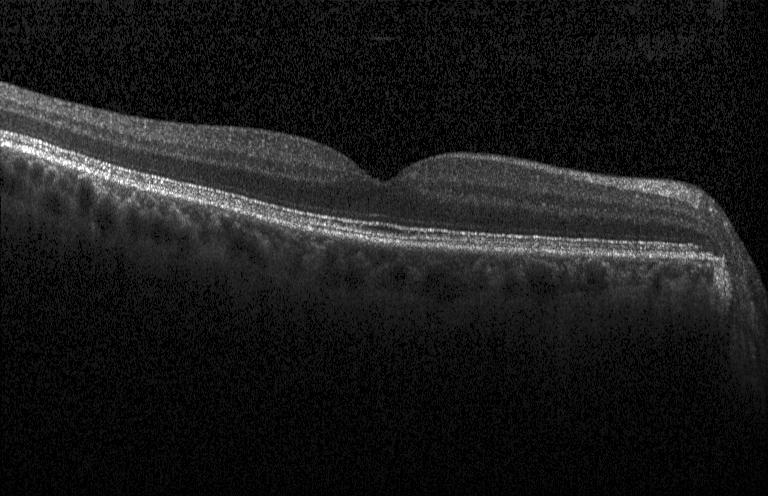

Retinal OCT B-scan · horizontal scan through the fovea — Finding: no choroidal neovascularization, no diabetic macular edema, and no drusen.